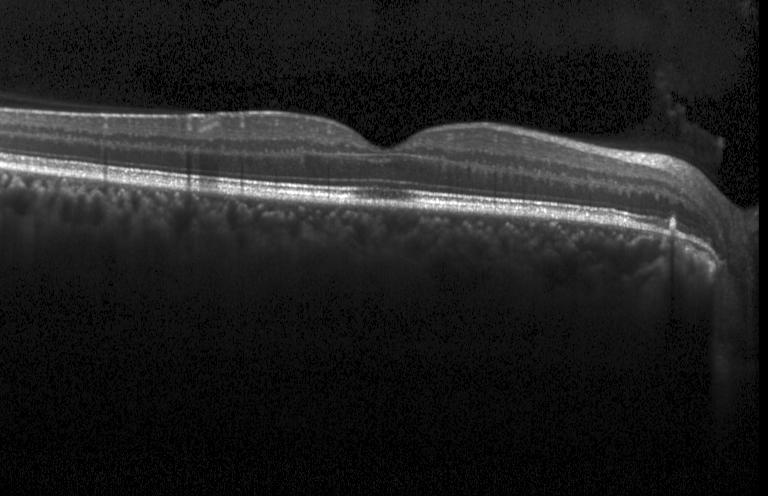

Through the macula · OCT line scan · spectral-domain OCT · acquired on a Heidelberg Spectralis — The scan shows neither CNV, DME, nor drusen.